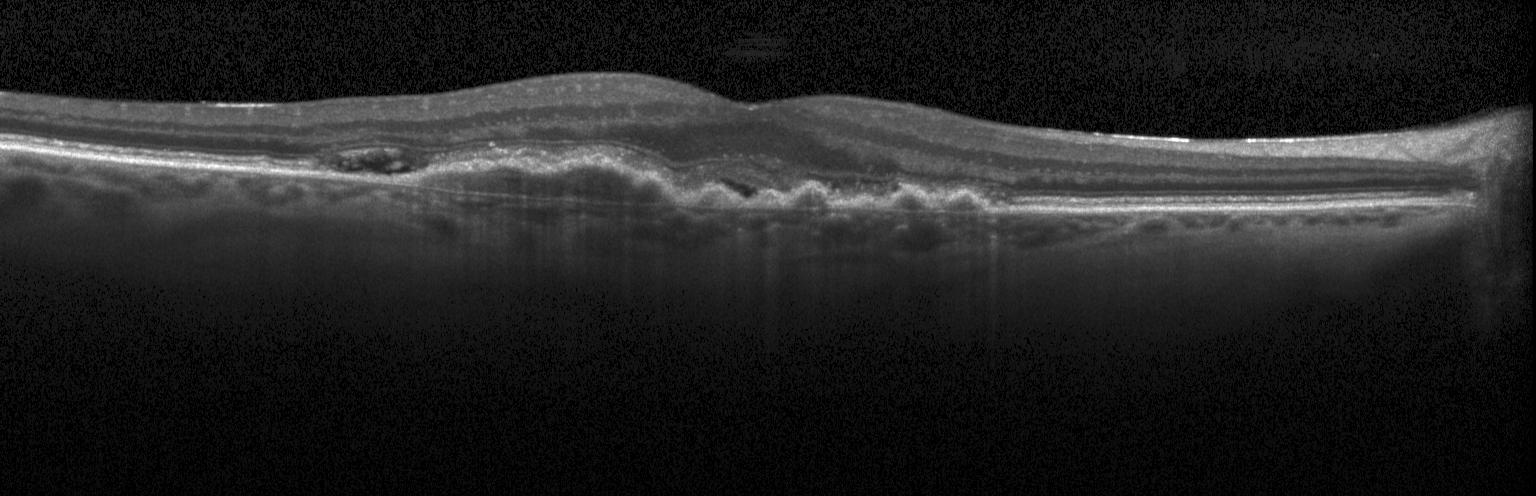

Instrument: Heidelberg Spectralis; OCT B-scan; macular scan; SD-OCT.
Finding: choroidal neovascularization.